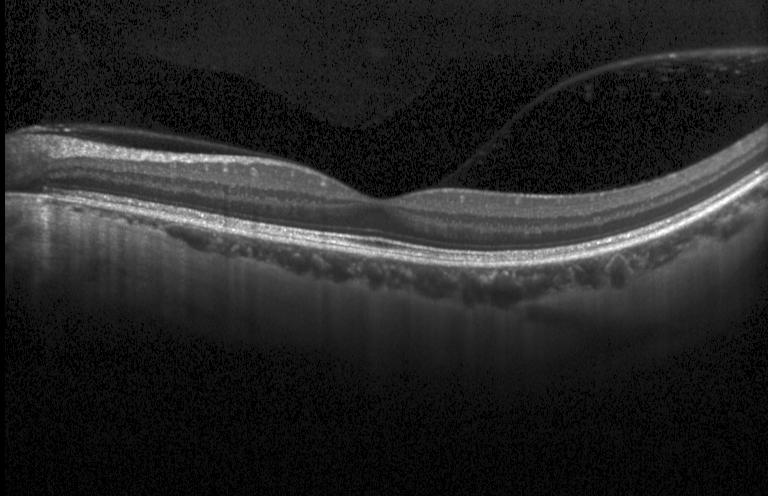

Centered on the fovea · acquired on a Heidelberg Spectralis · optical coherence tomography B-scan
Assessment: no evidence of choroidal neovascularization, diabetic macular edema, or drusen.